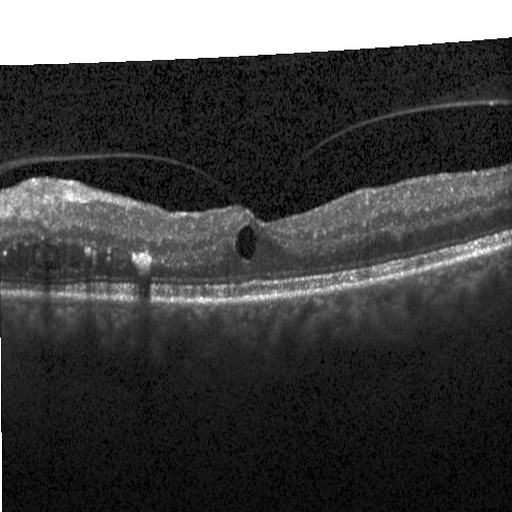

Spectral-domain optical coherence tomography; macular scan; OCT B-scan; acquired on a Heidelberg Spectralis — Macular OCT: diabetic macular edema (DME).